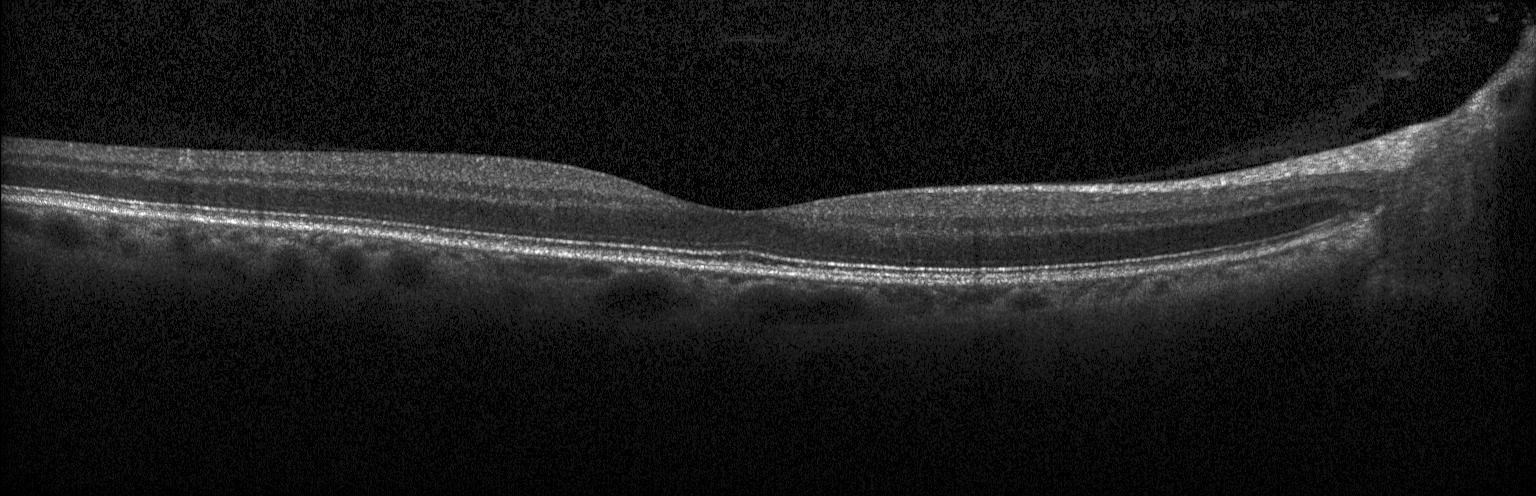

OCT line scan. Impression: no evidence of choroidal neovascularization, diabetic macular edema, or drusen.